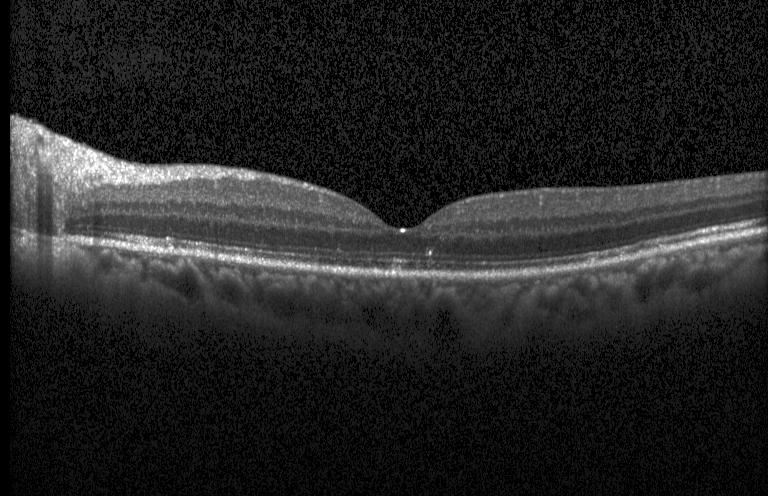

Impression: no evidence of choroidal neovascularization, diabetic macular edema, or drusen.